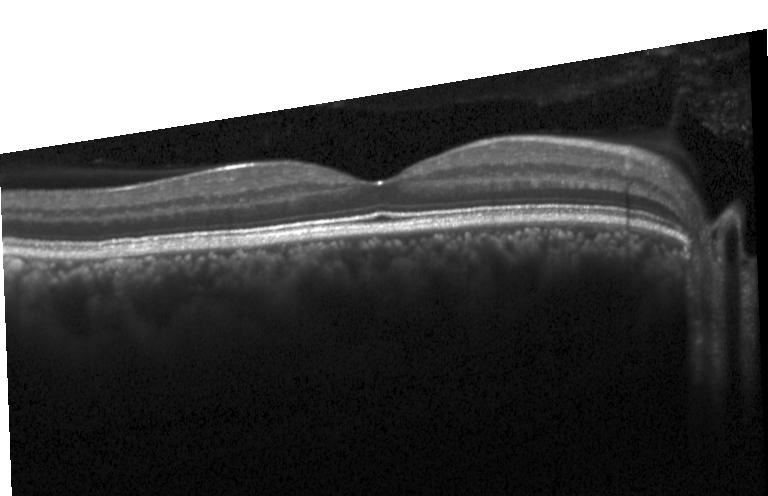

Optical coherence tomography B-scan.
Impression: no evidence of choroidal neovascularization, diabetic macular edema, or drusen.